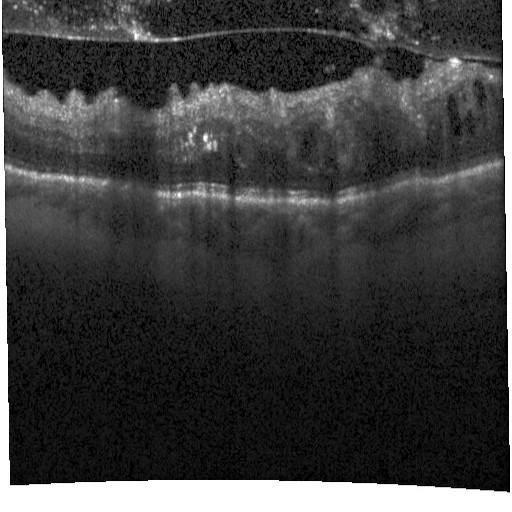 Impression: diabetic macular edema.